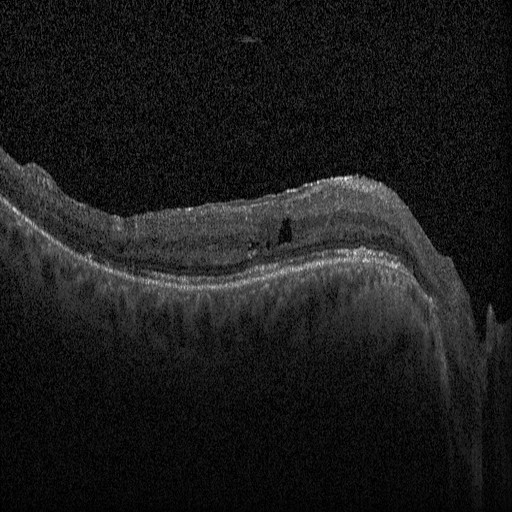

OCT B-scan; SD-OCT.
Finding: DME.